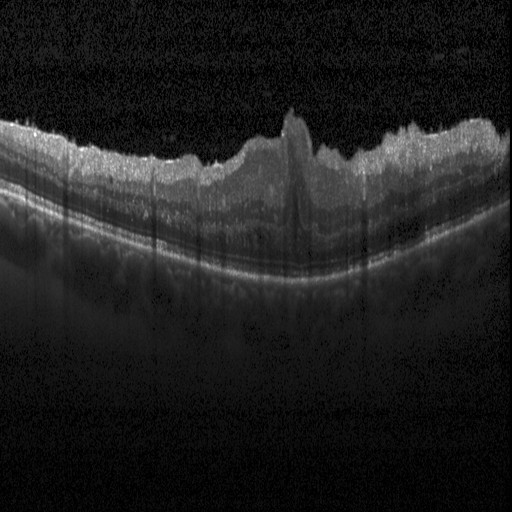 Fovea-centered, spectral-domain OCT, optical coherence tomography scan, acquired on a Heidelberg Spectralis
The scan shows diabetic macular edema.